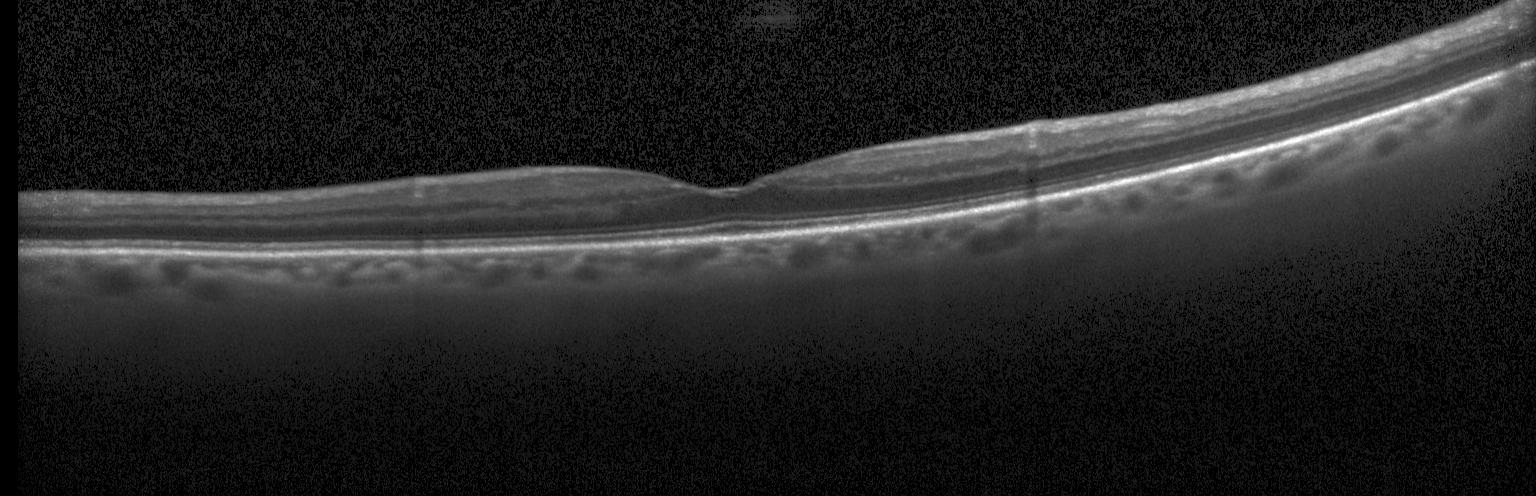

Heidelberg Spectralis OCT system; optical coherence tomography scan. Diagnosis: neither choroidal neovascularization, diabetic macular edema, nor drusen.